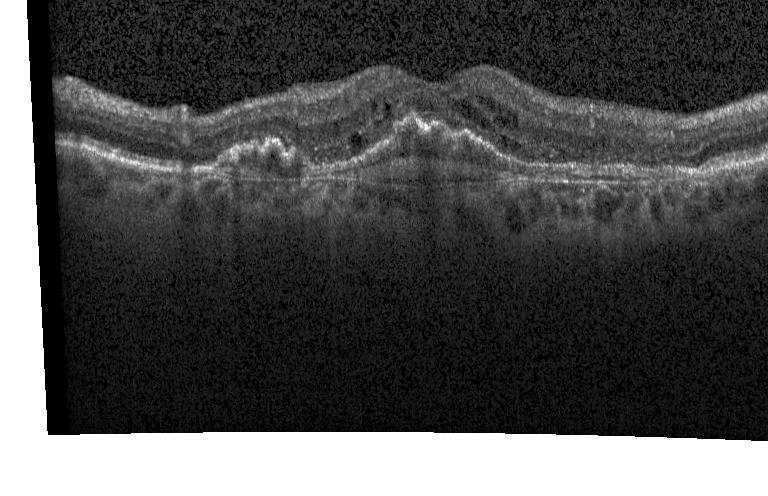 Macular OCT demonstrating a choroidal neovascular membrane.